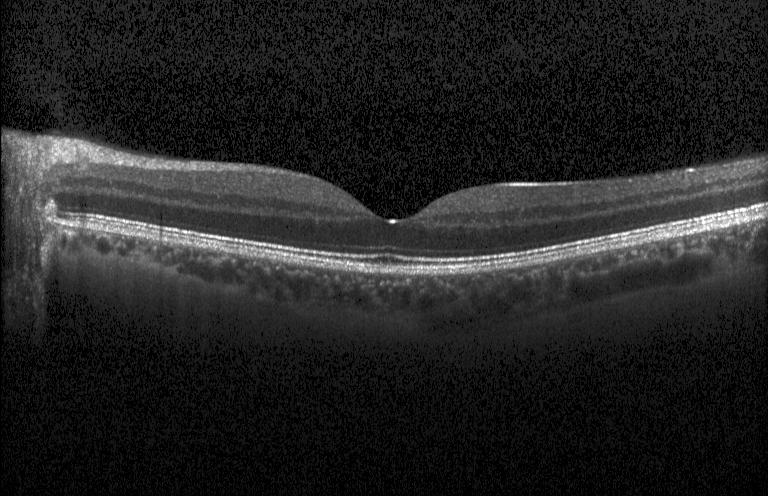
Retinal OCT B-scan. Macular OCT: no choroidal neovascularization, diabetic macular edema, or drusen.